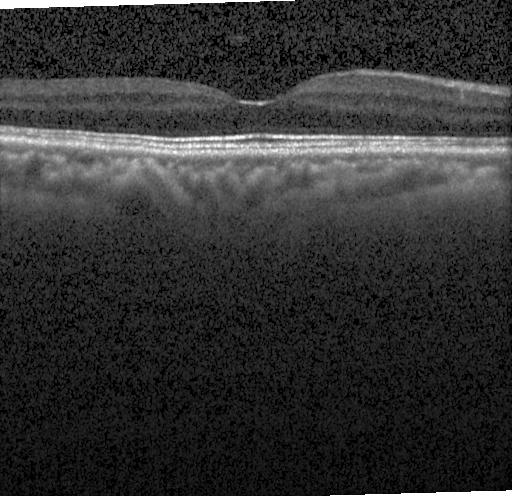 Macular OCT: no choroidal neovascularization, no diabetic macular edema, and no drusen.